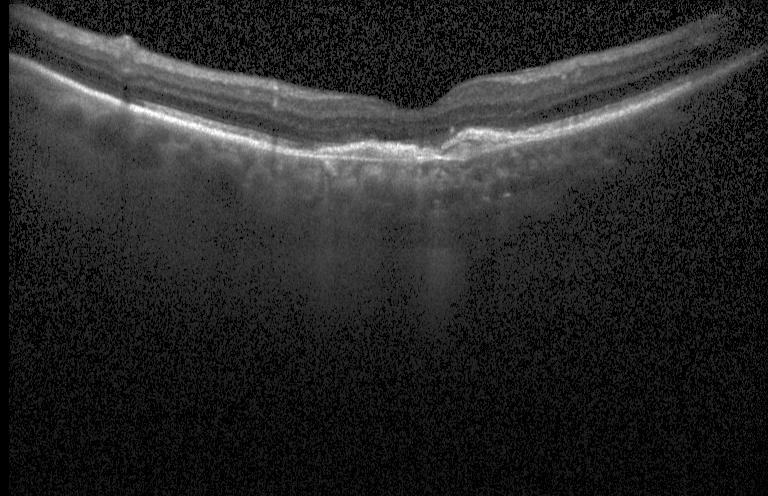

Diagnosis: choroidal neovascularization.